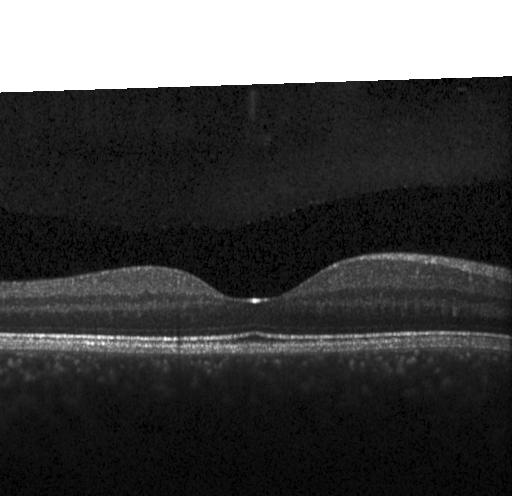

OCT finding: no CNV, no DME, and no drusen.